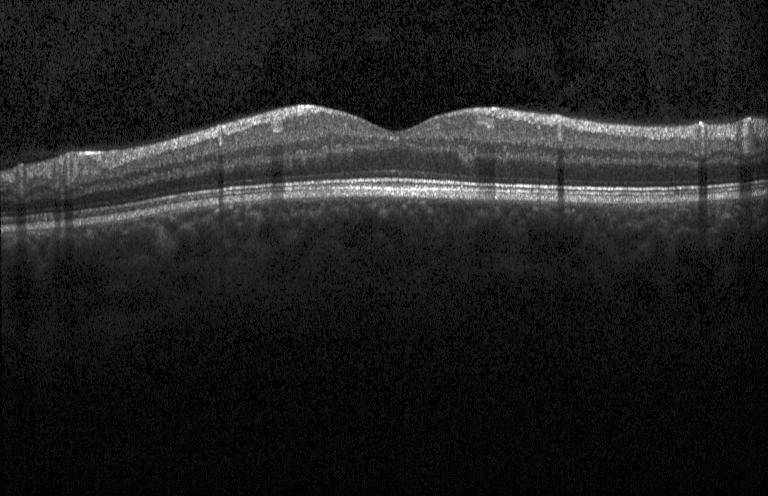

Impression: neither CNV, DME, nor drusen.